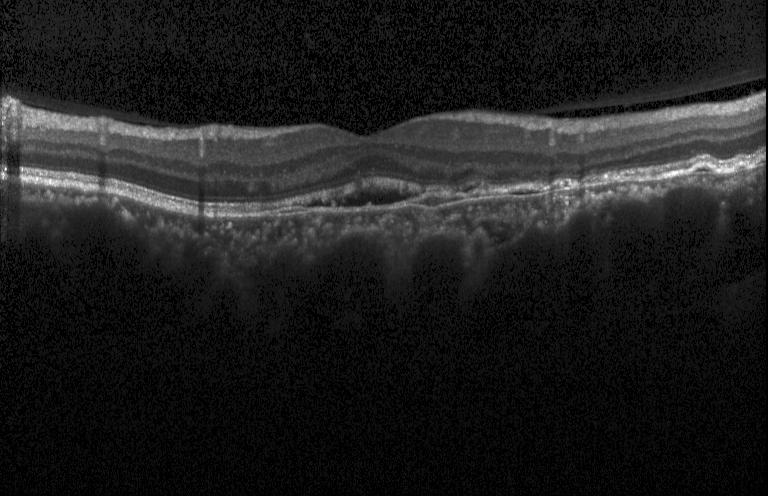 Dx: CNV.